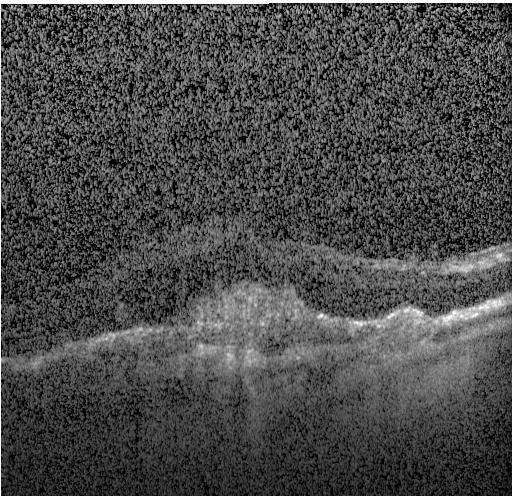 Retinal OCT cross-section showing a choroidal neovascular membrane.